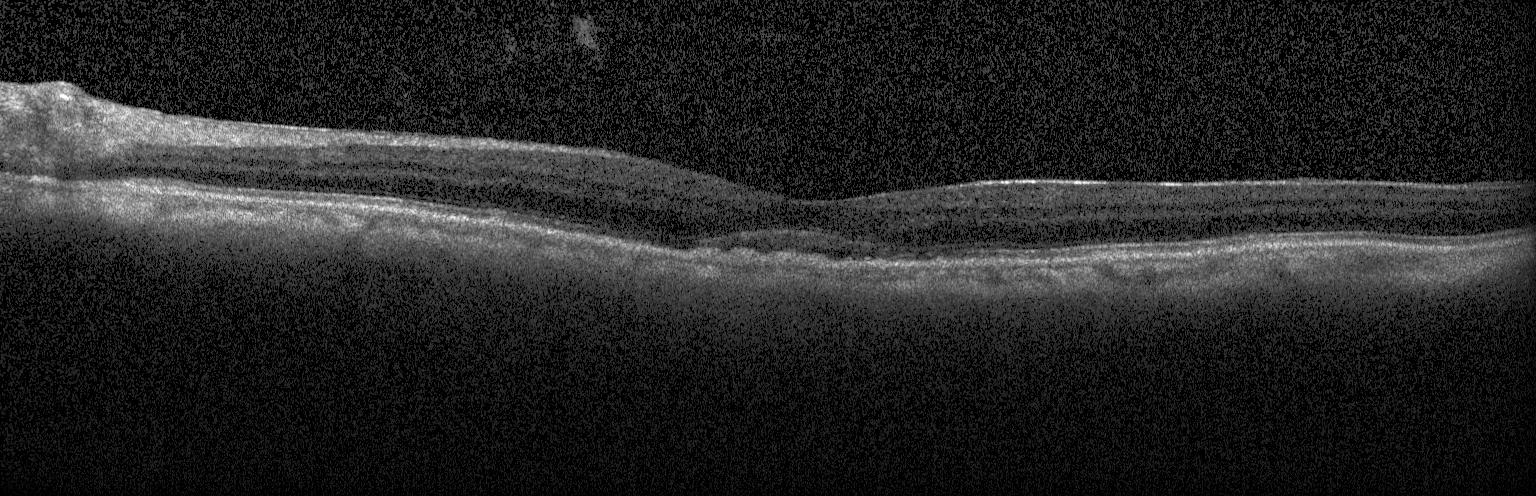 Diagnosis: choroidal neovascularization (CNV).